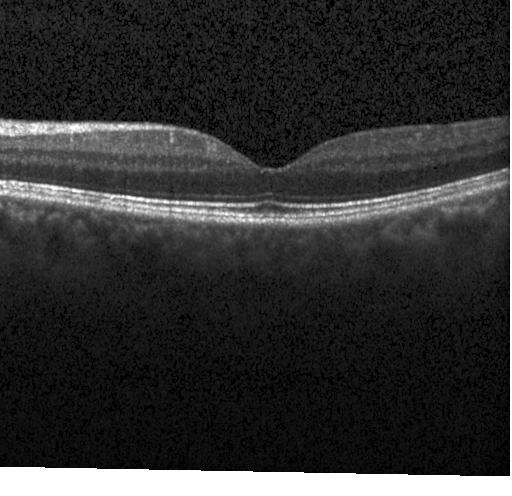 Optical coherence tomography scan. Macular scan. Dx: no evidence of choroidal neovascularization, diabetic macular edema, or drusen.